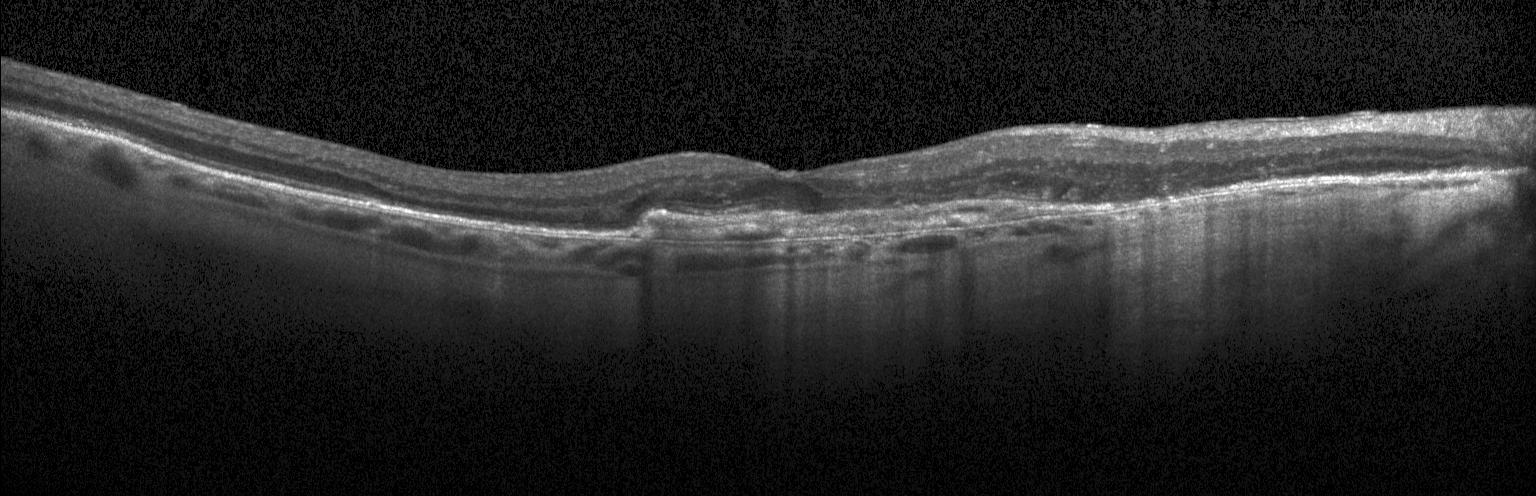
This B-scan demonstrates a choroidal neovascular membrane.